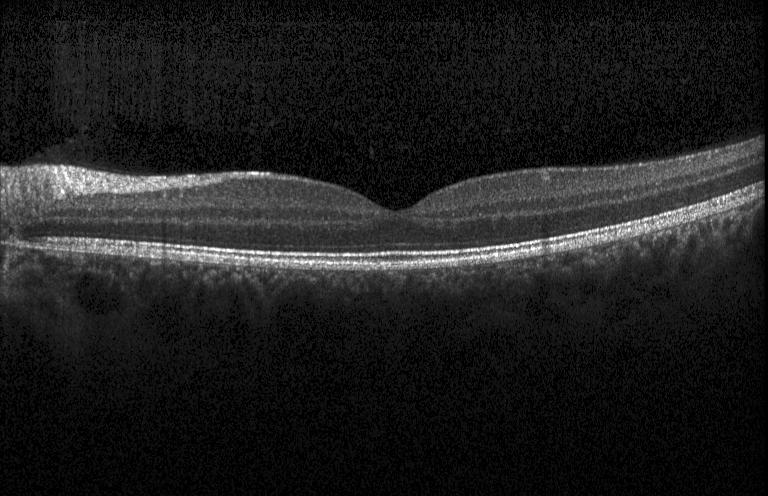
Retinal OCT cross-section. Centered on the fovea. SD-OCT.
This B-scan demonstrates neither CNV, DME, nor drusen.